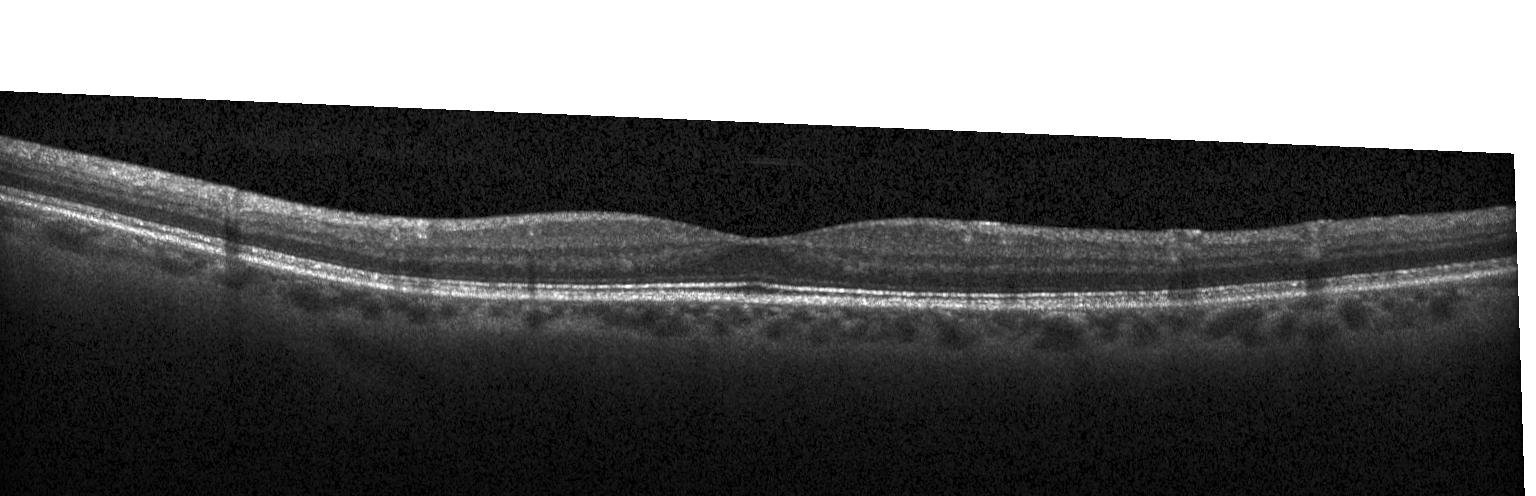

Instrument: Heidelberg Spectralis; optical coherence tomography B-scan; centered on the fovea.
Diagnosis: no choroidal neovascularization, diabetic macular edema, or drusen.